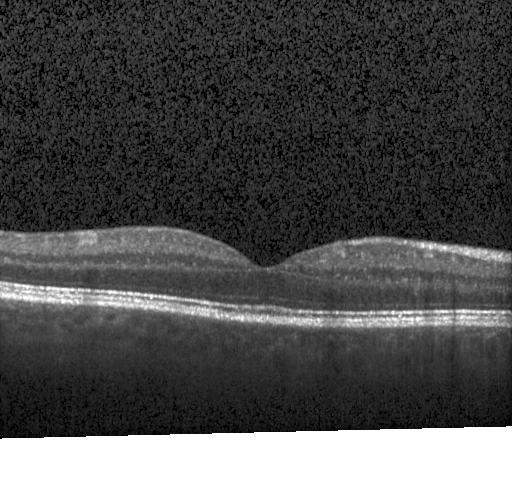

Optical coherence tomography scan.
Dx: no choroidal neovascularization, diabetic macular edema, or drusen.